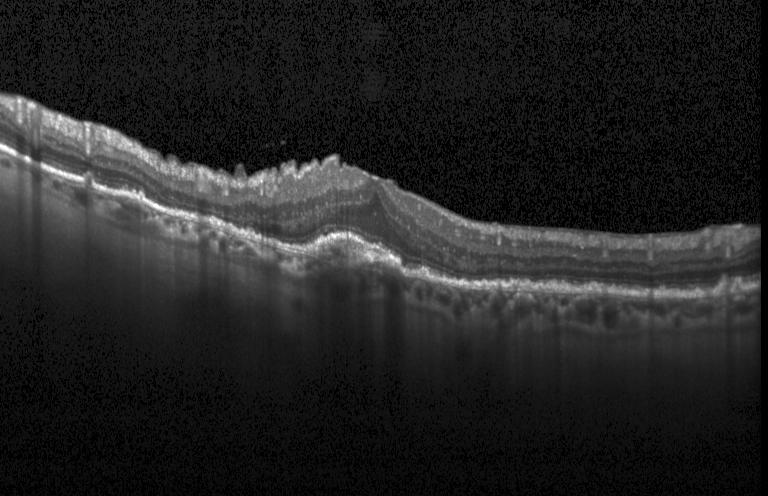
Macular OCT demonstrating a choroidal neovascular membrane.